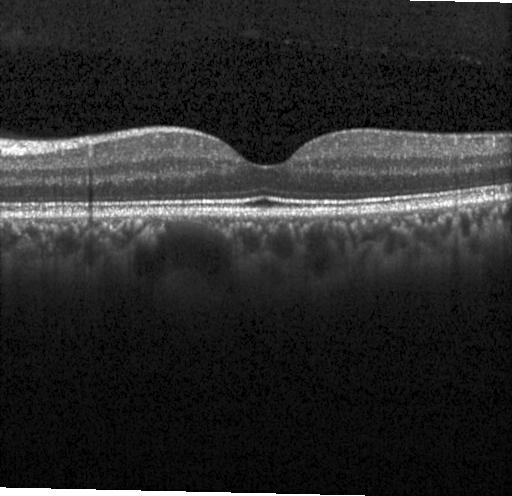

Spectral-domain OCT B-scan: no choroidal neovascularization, diabetic macular edema, or drusen.